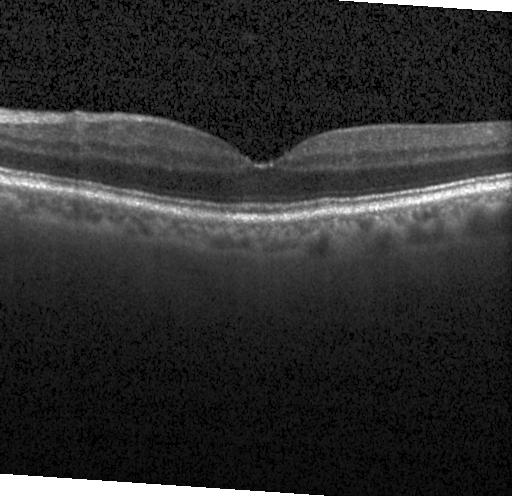

Retinal OCT cross-section · Heidelberg Spectralis · spectral-domain optical coherence tomography. Finding: no choroidal neovascularization, diabetic macular edema, or drusen.